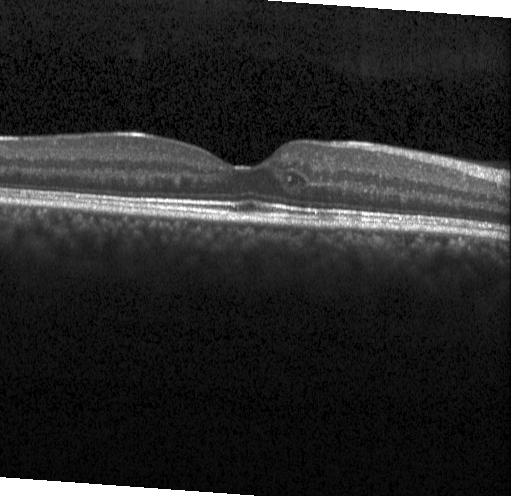

Spectral-domain OCT · fovea-centered · OCT B-scan · instrument: Heidelberg Spectralis. Diagnosis: diabetic macular edema.